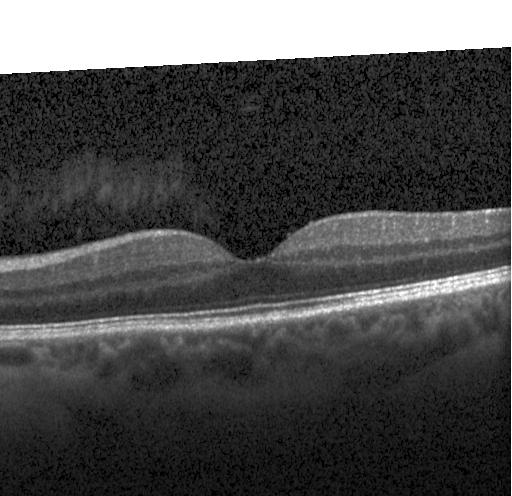

Impression: no choroidal neovascularization, no diabetic macular edema, and no drusen.